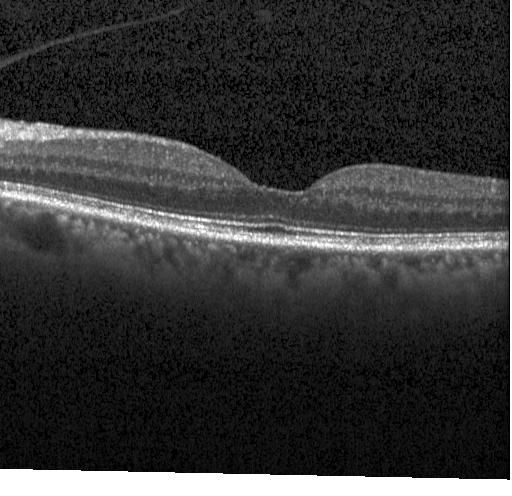
Retinal OCT cross-section · instrument: Heidelberg Spectralis — This B-scan demonstrates no choroidal neovascularization, no diabetic macular edema, and no drusen.